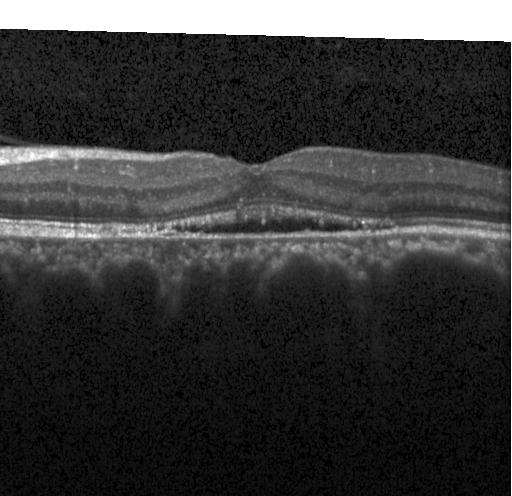 Macular OCT demonstrating a choroidal neovascular membrane.